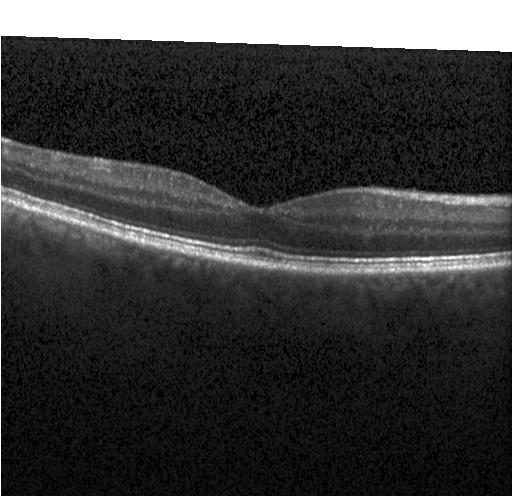

Diagnosis: neither choroidal neovascularization, diabetic macular edema, nor drusen.